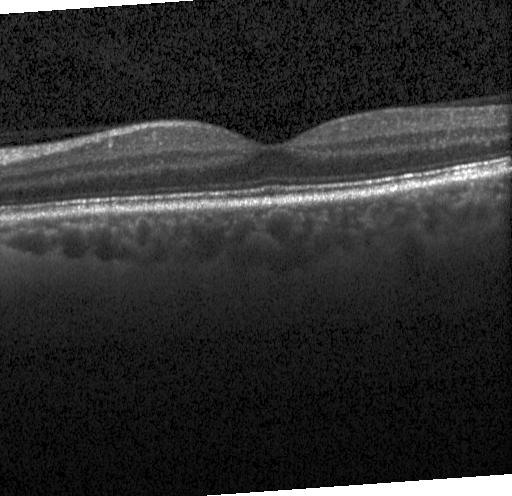
Finding: no choroidal neovascularization, no diabetic macular edema, and no drusen.